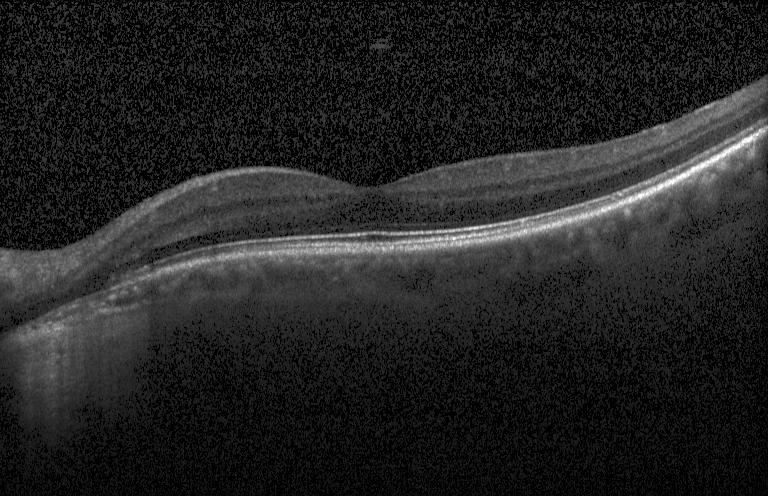
Macular OCT demonstrating no CNV, DME, or drusen.